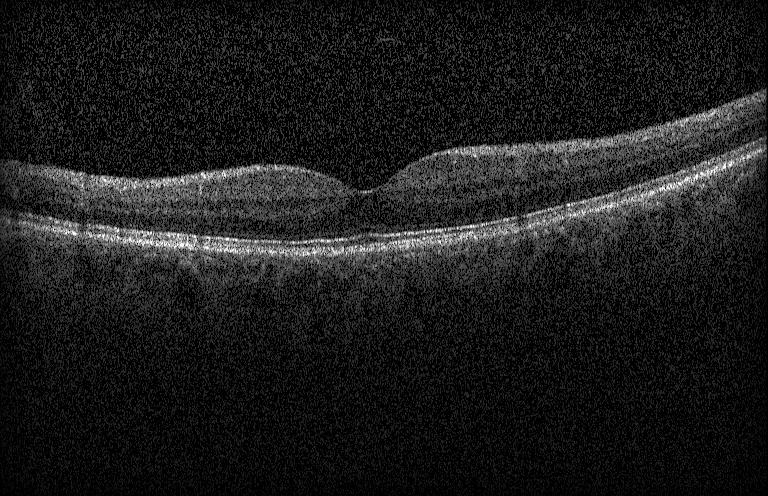
Optical coherence tomography B-scan
Finding: no choroidal neovascularization, diabetic macular edema, or drusen.